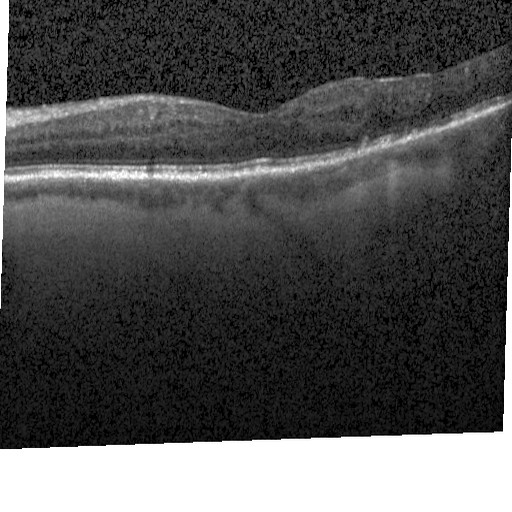

OCT scan showing diabetic macular edema.